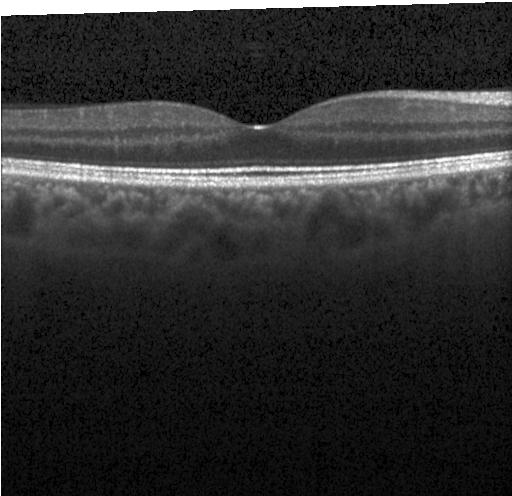
Finding: neither choroidal neovascularization, diabetic macular edema, nor drusen.